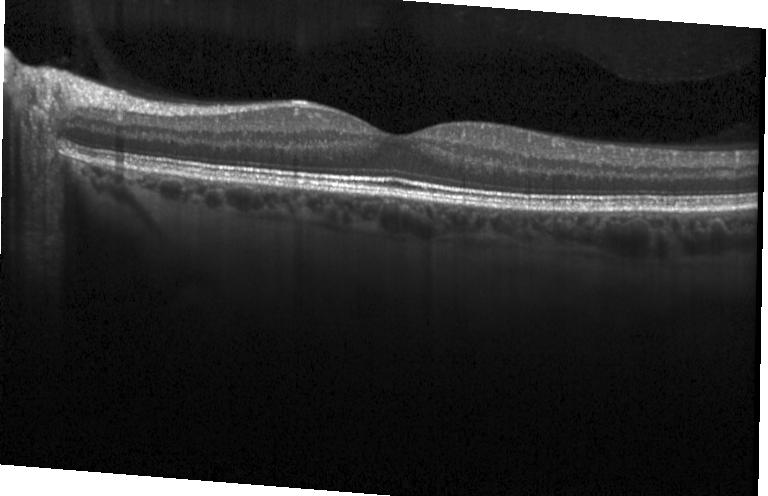

SD-OCT. Fovea-centered. Instrument: Heidelberg Spectralis. Retinal OCT B-scan
Impression: no evidence of choroidal neovascularization, diabetic macular edema, or drusen.